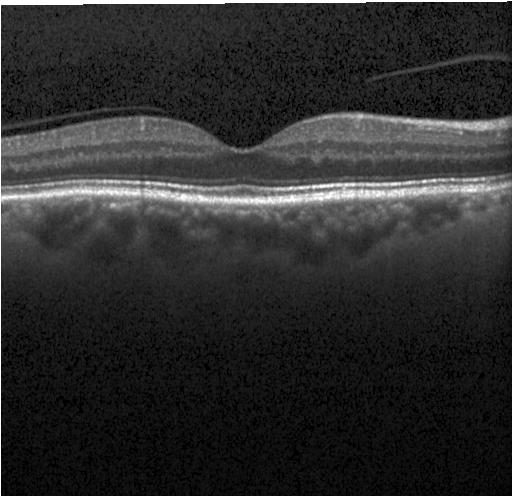

OCT B-scan; horizontal scan through the fovea — Dx: neither choroidal neovascularization, diabetic macular edema, nor drusen.